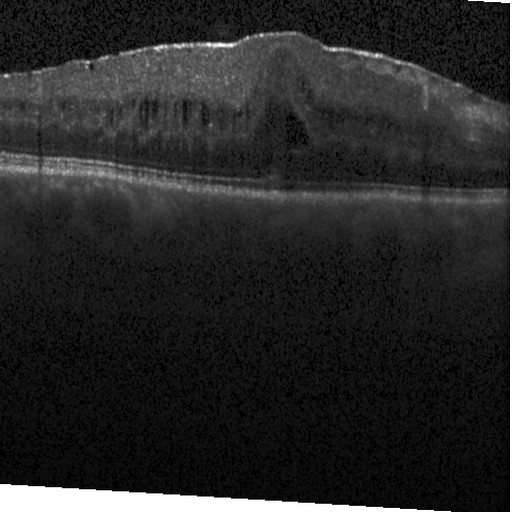

Macular OCT demonstrating DME.